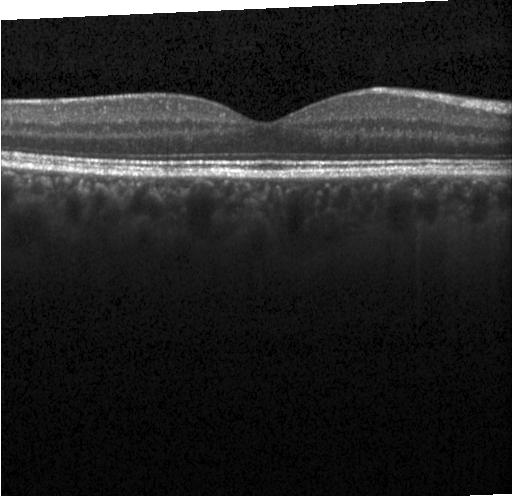

OCT finding: no evidence of choroidal neovascularization, diabetic macular edema, or drusen.